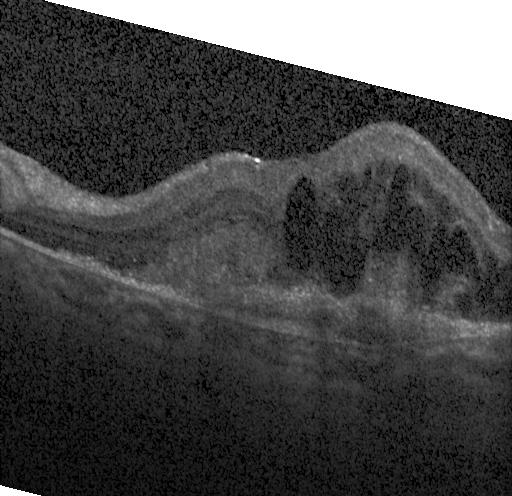
Macular OCT: a choroidal neovascular membrane.